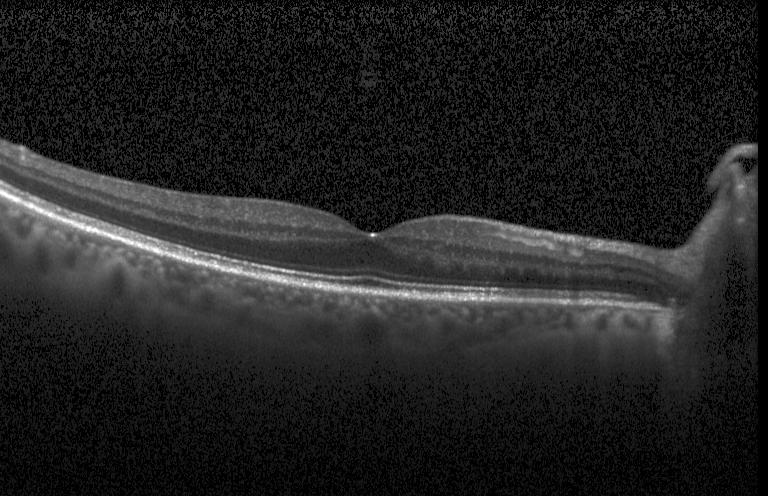
OCT B-scan; spectral-domain optical coherence tomography. Macular OCT: no evidence of CNV, DME, or drusen.